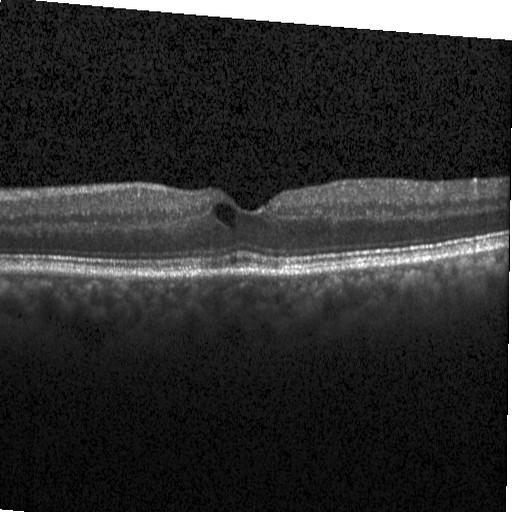 Assessment: diabetic macular edema.